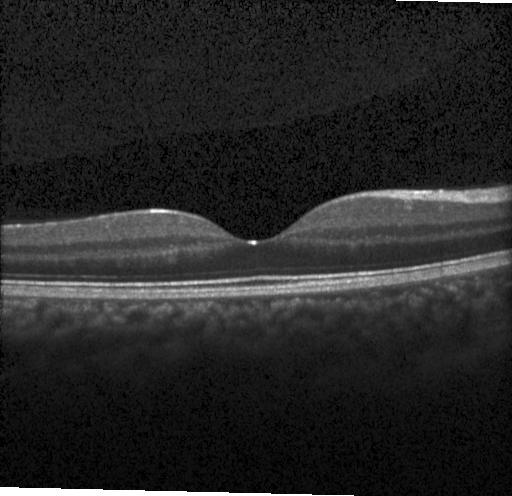

Acquired on a Heidelberg Spectralis, spectral-domain OCT, retinal OCT B-scan.
Dx: no CNV, DME, or drusen.